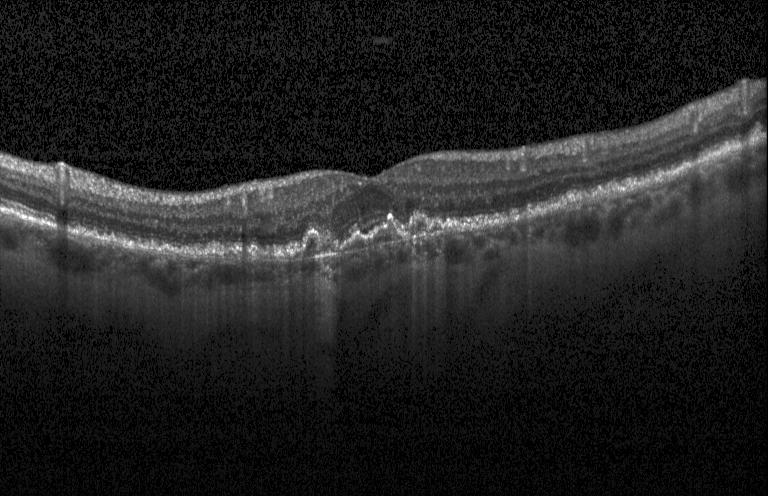

Optical coherence tomography scan; SD-OCT; Heidelberg Spectralis; horizontal scan through the fovea.
Assessment: a choroidal neovascular membrane.